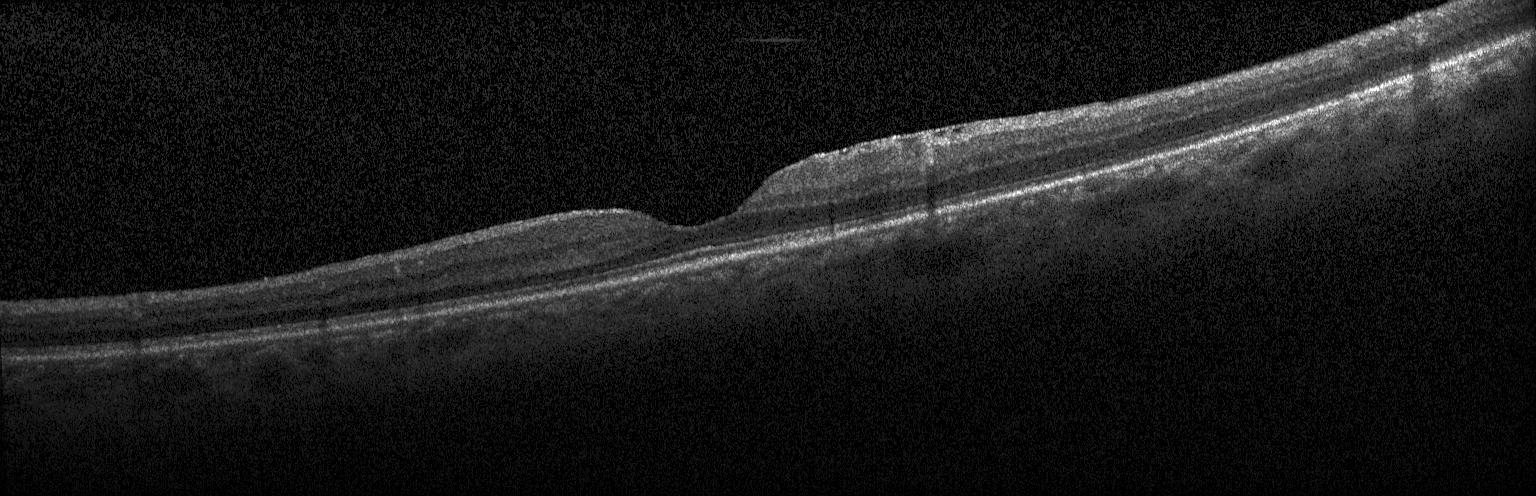 Retinal OCT B-scan
No choroidal neovascularization, diabetic macular edema, or drusen.